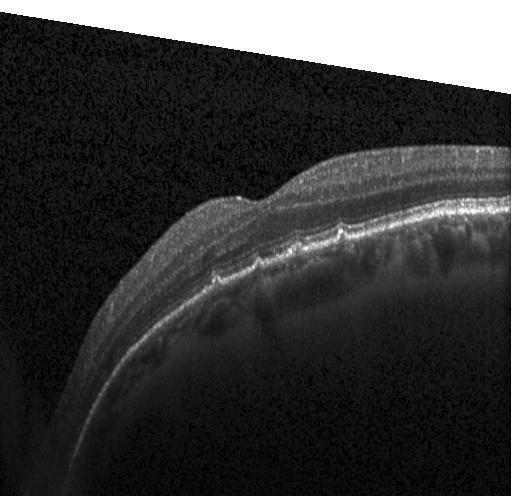
Impression: sub-RPE drusenoid deposits.